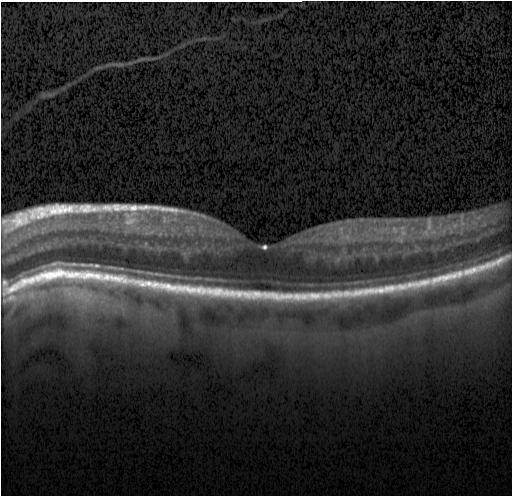
OCT B-scan.
Diagnosis: no choroidal neovascularization, no diabetic macular edema, and no drusen.